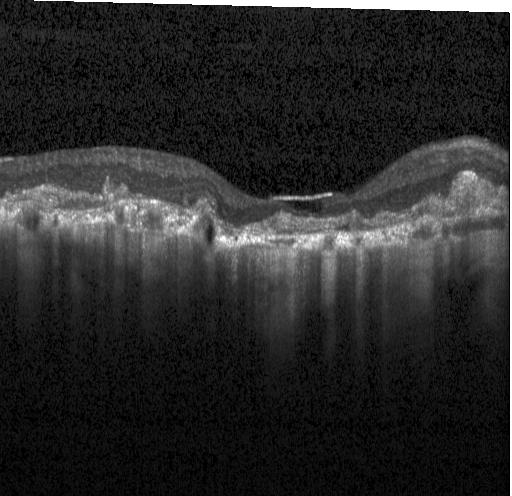 Retinal OCT B-scan. Fovea-centered — A choroidal neovascular membrane.